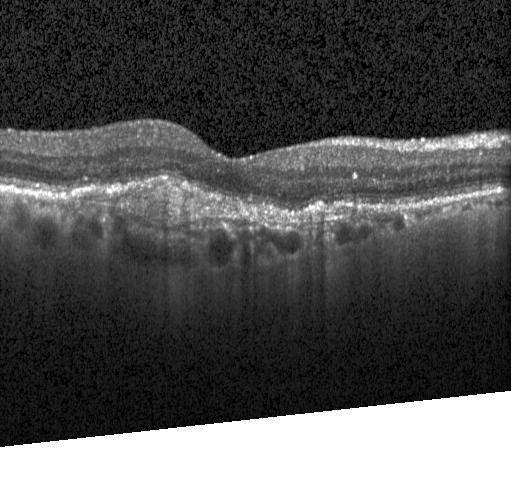 Retinal OCT cross-section · spectral-domain optical coherence tomography · fovea-centered
OCT finding: a choroidal neovascular membrane.